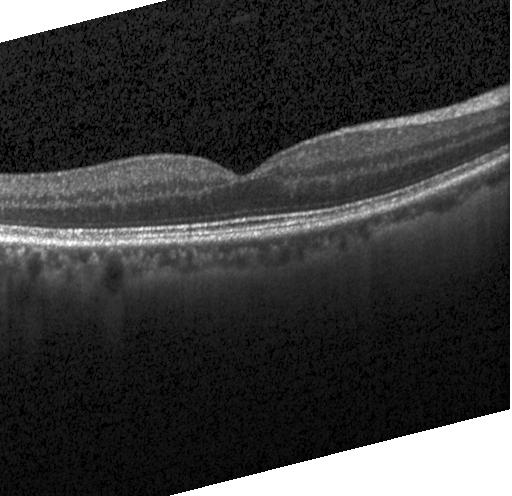

OCT line scan; spectral-domain optical coherence tomography; centered on the fovea. Macular OCT: no choroidal neovascularization, diabetic macular edema, or drusen.